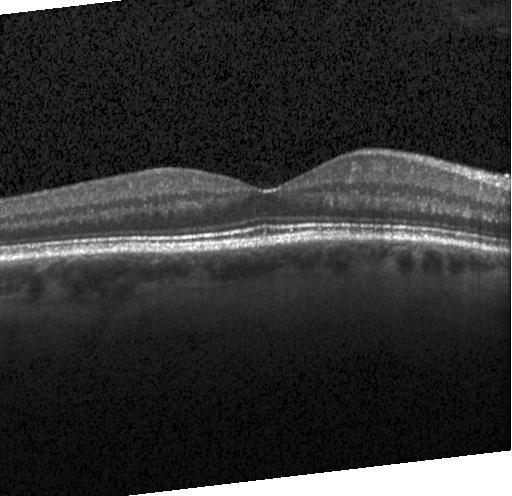
This B-scan demonstrates no choroidal neovascularization, diabetic macular edema, or drusen.